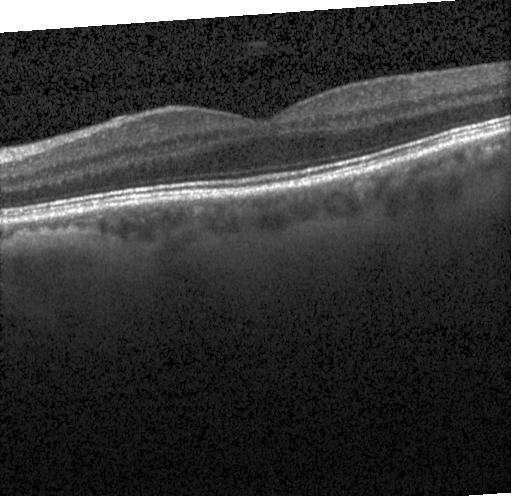
SD-OCT. OCT line scan. Horizontal scan through the fovea.
Diagnosis: neither choroidal neovascularization, diabetic macular edema, nor drusen.